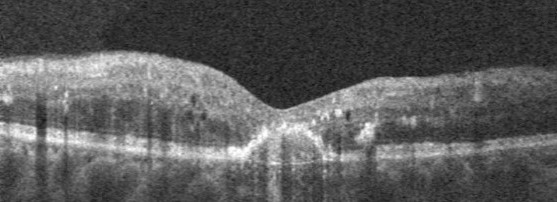

The scan shows diabetic macular edema (DME).